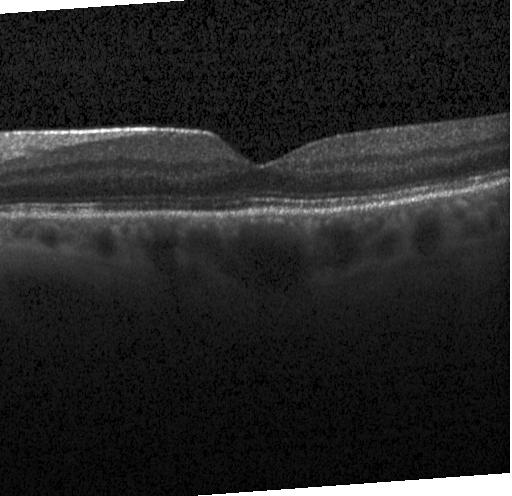 Spectral-domain optical coherence tomography · retinal OCT B-scan — Impression: no CNV, no DME, and no drusen.